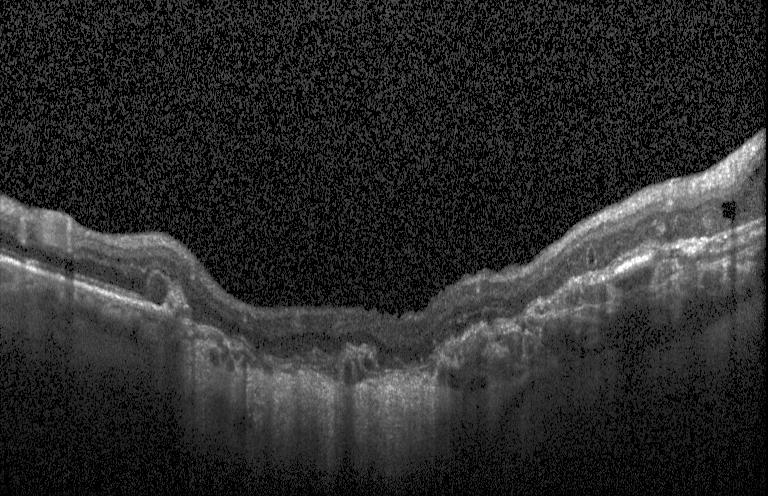
Finding: CNV.